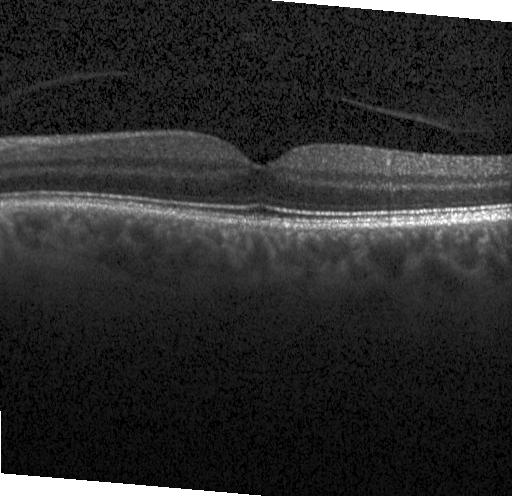
Retinal OCT cross-section showing no CNV, DME, or drusen.